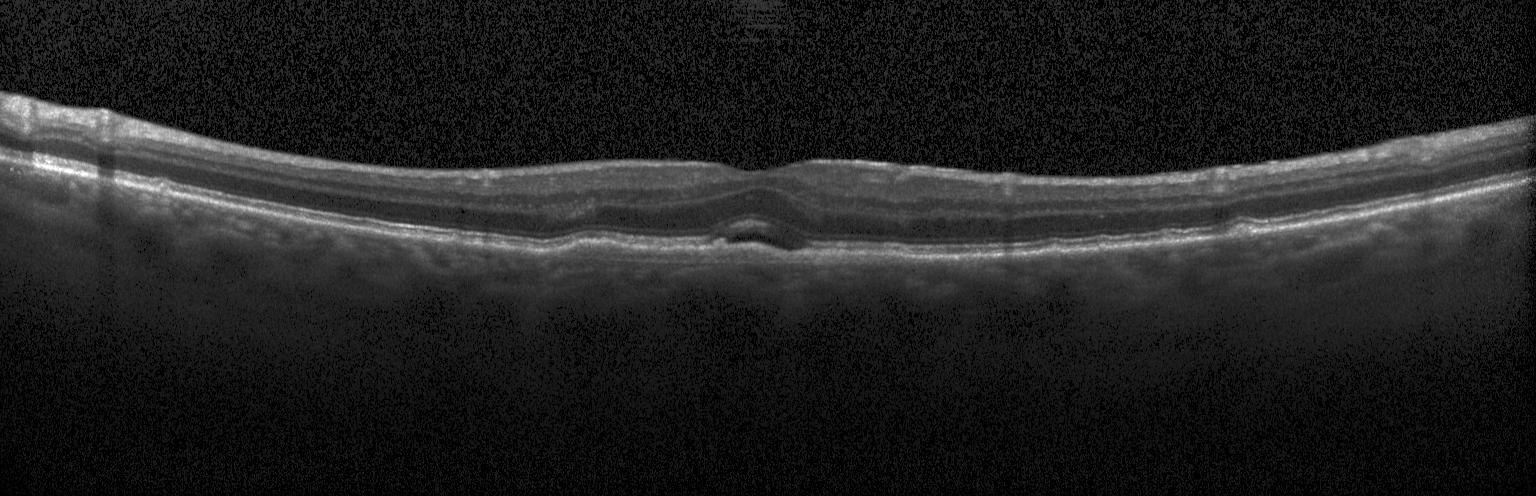

Centered on the fovea; retinal OCT B-scan; spectral-domain optical coherence tomography; acquired on a Heidelberg Spectralis
Diagnosis: a choroidal neovascular membrane.